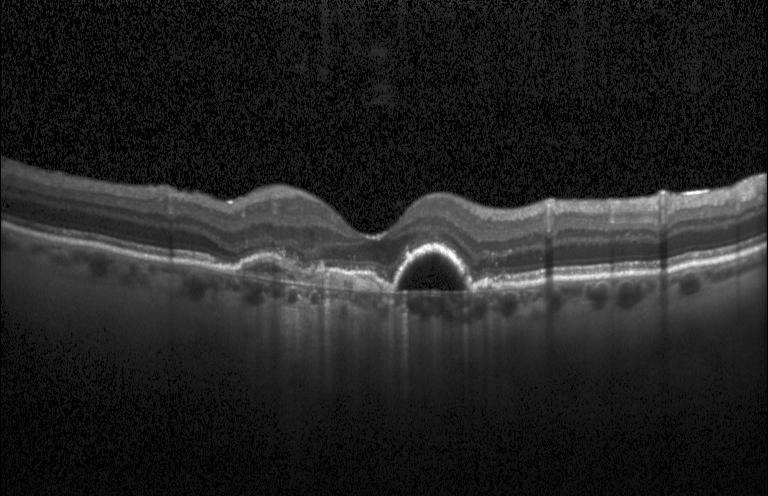
Retinal OCT cross-section · horizontal scan through the fovea · spectral-domain optical coherence tomography
Macular OCT: CNV.